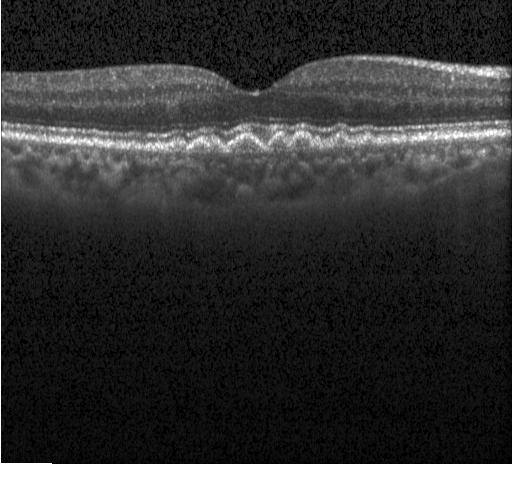
OCT finding: multiple drusen.